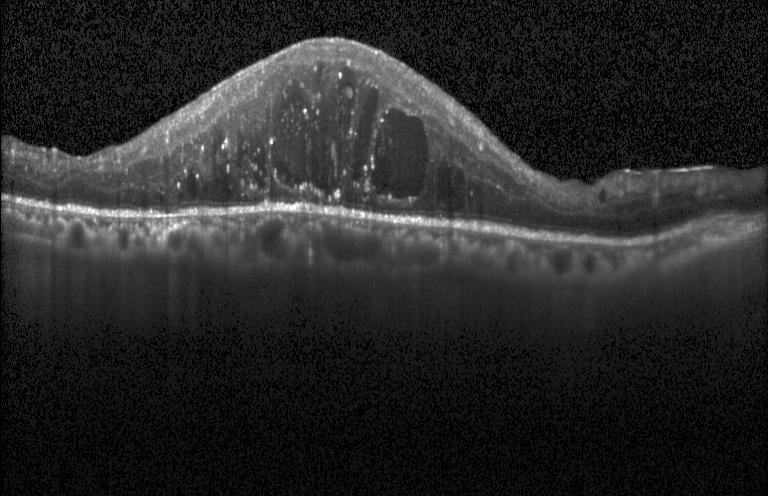

Diagnosis: diabetic macular edema (DME).